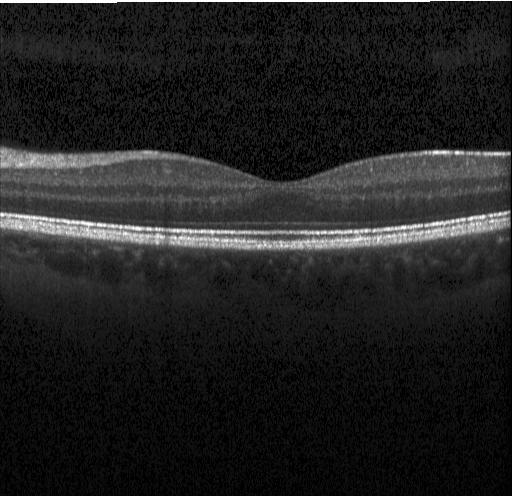
SD-OCT. Retinal OCT cross-section.
Finding: no choroidal neovascularization, diabetic macular edema, or drusen.